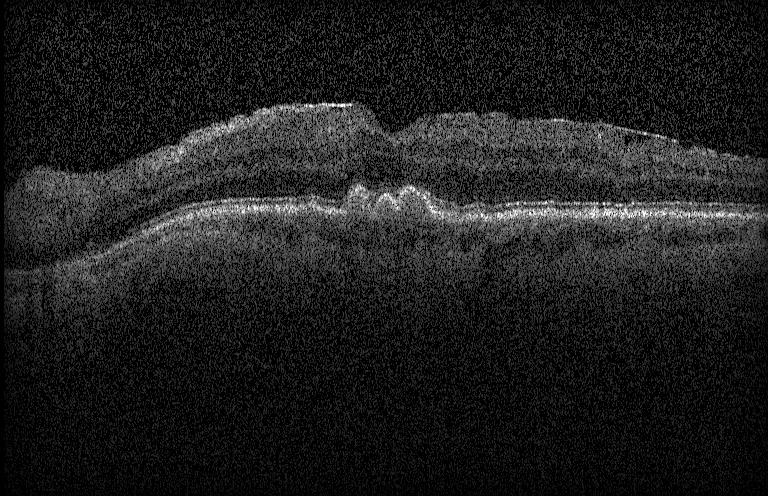

Through the macula; OCT line scan; spectral-domain OCT.
This B-scan demonstrates drusen.